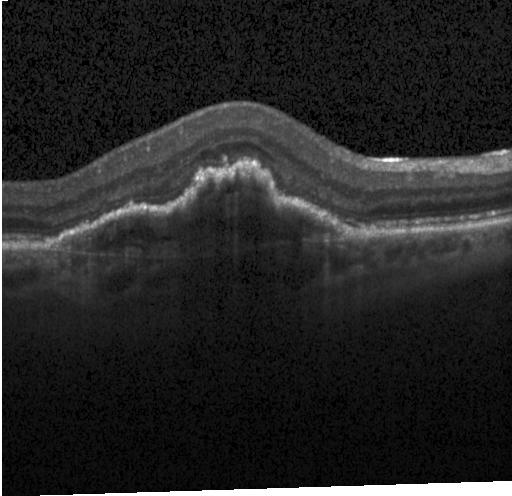 Impression: a choroidal neovascular membrane.